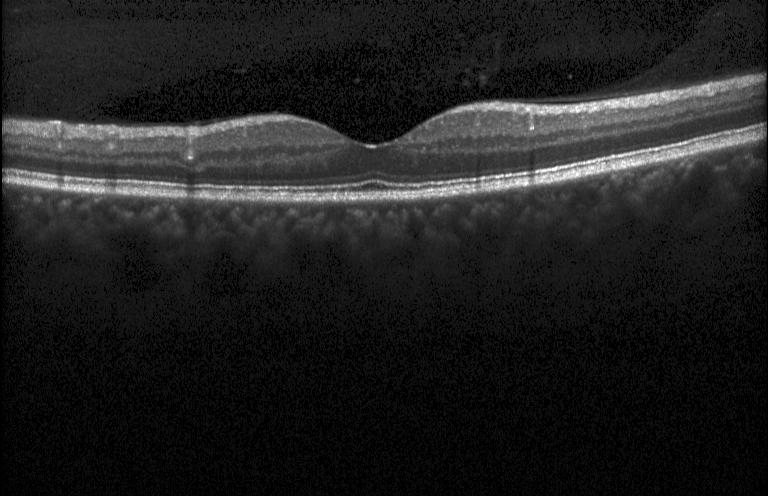 SD-OCT. Centered on the fovea. Retinal OCT B-scan. Instrument: Heidelberg Spectralis
The scan shows no choroidal neovascularization, diabetic macular edema, or drusen.